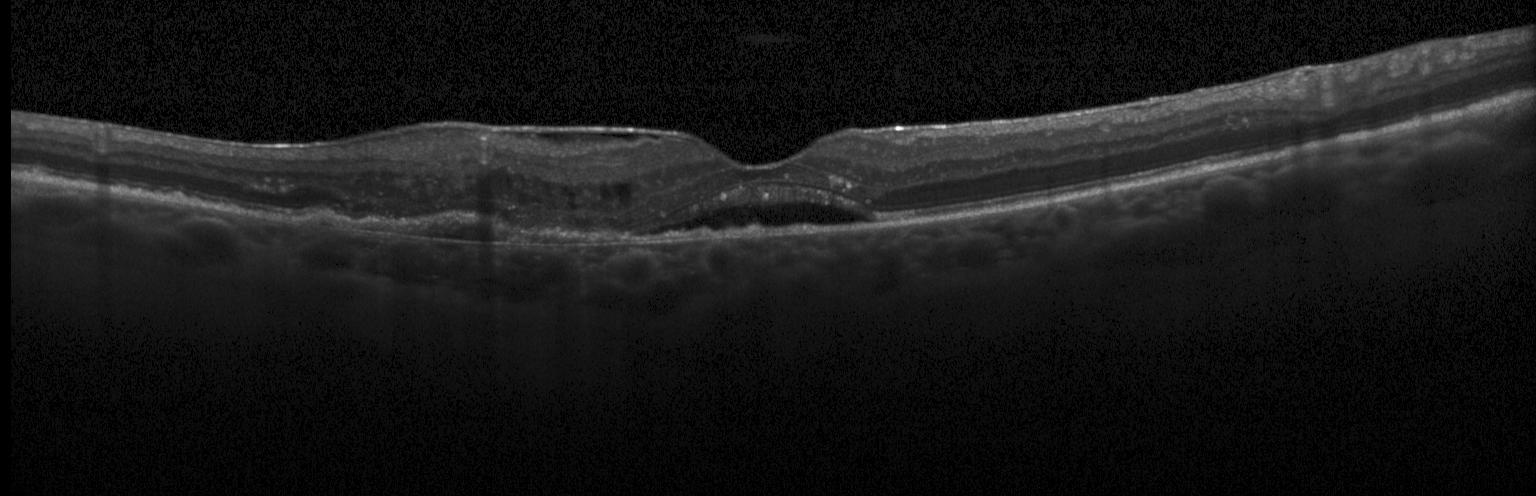
Finding: a choroidal neovascular membrane.